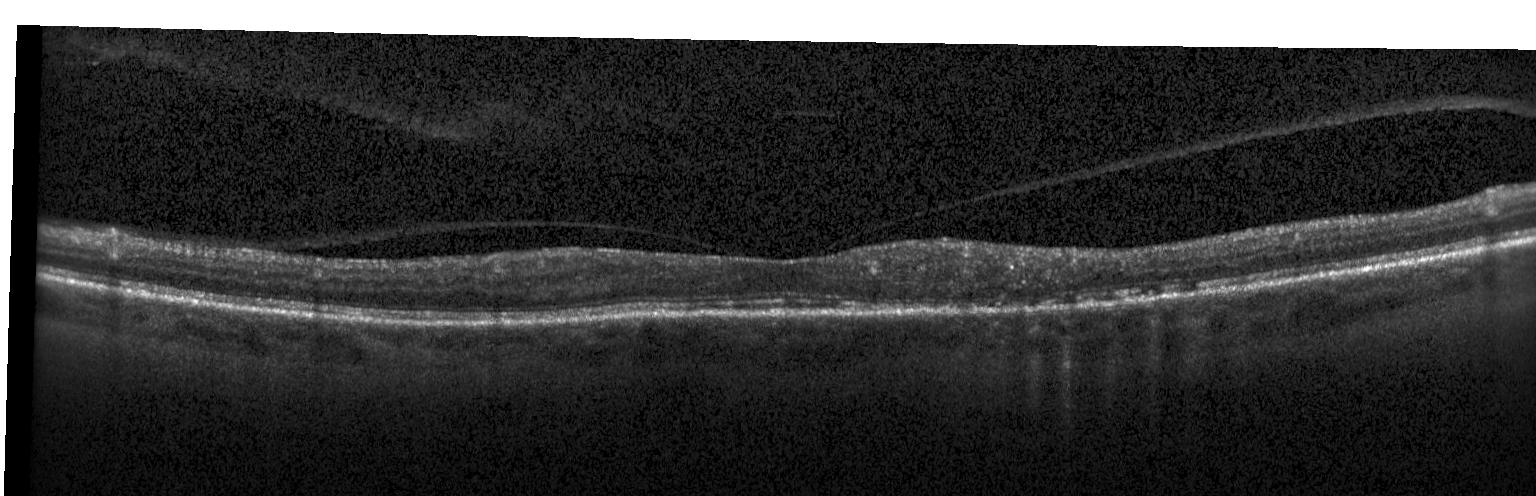
SD-OCT, retinal OCT cross-section — Finding: DME.